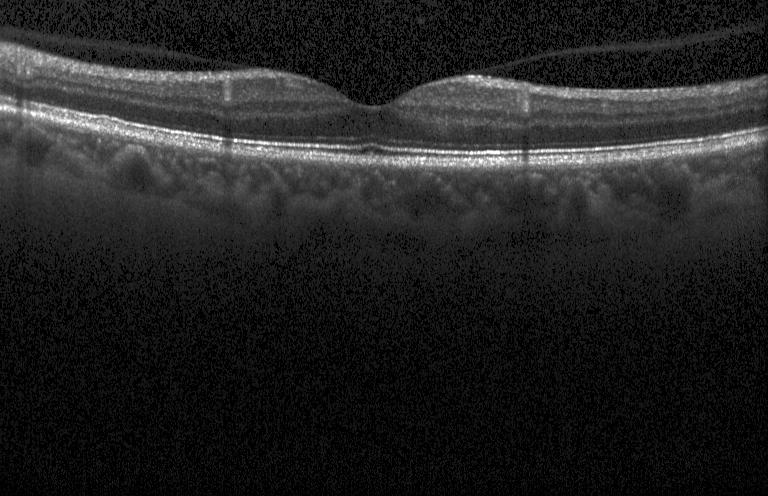
Optical coherence tomography scan; centered on the fovea.
OCT finding: no CNV, DME, or drusen.